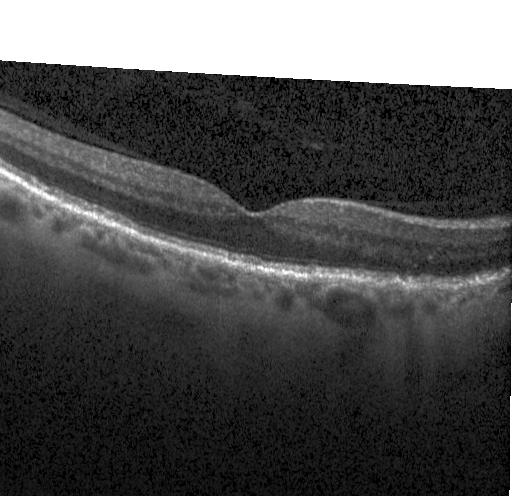 Spectral-domain OCT · OCT B-scan · through the macula
Impression: no CNV, DME, or drusen.